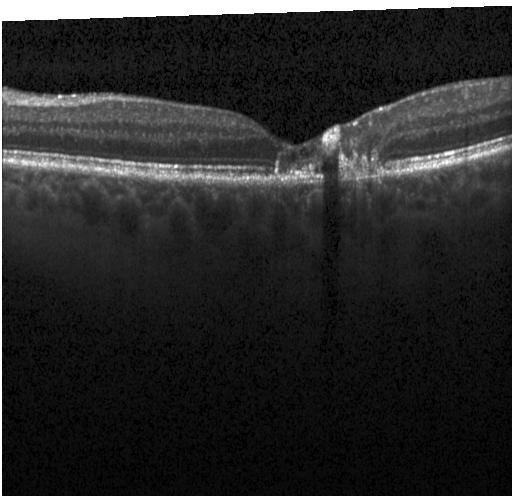

Instrument: Heidelberg Spectralis, spectral-domain optical coherence tomography, OCT line scan — Finding: a choroidal neovascular membrane.